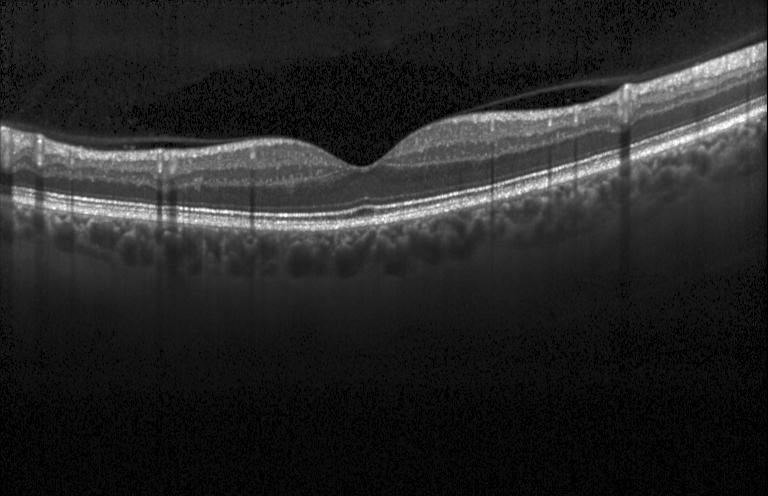 Optical coherence tomography B-scan
Impression: no choroidal neovascularization, no diabetic macular edema, and no drusen.